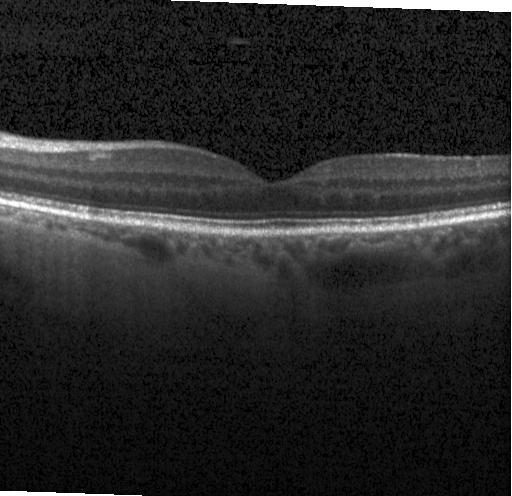
Heidelberg Spectralis OCT system, optical coherence tomography B-scan, spectral-domain optical coherence tomography, centered on the fovea
Finding: no CNV, DME, or drusen.